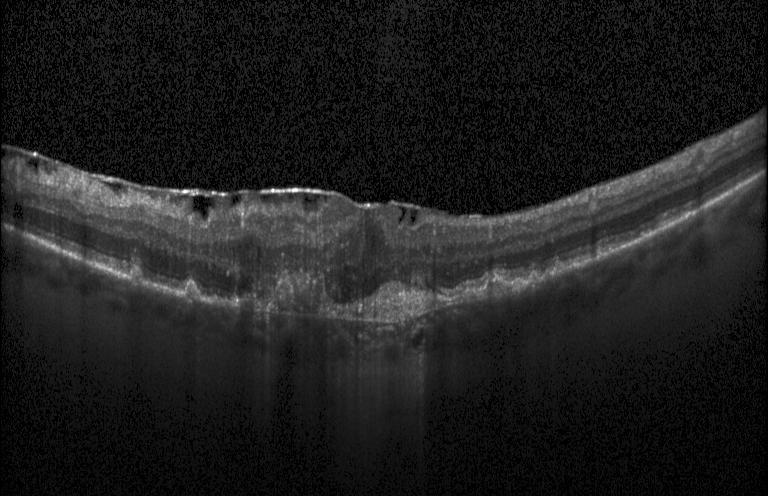 Optical coherence tomography scan; instrument: Heidelberg Spectralis; spectral-domain optical coherence tomography; horizontal scan through the fovea.
Diagnosis: a choroidal neovascular membrane.